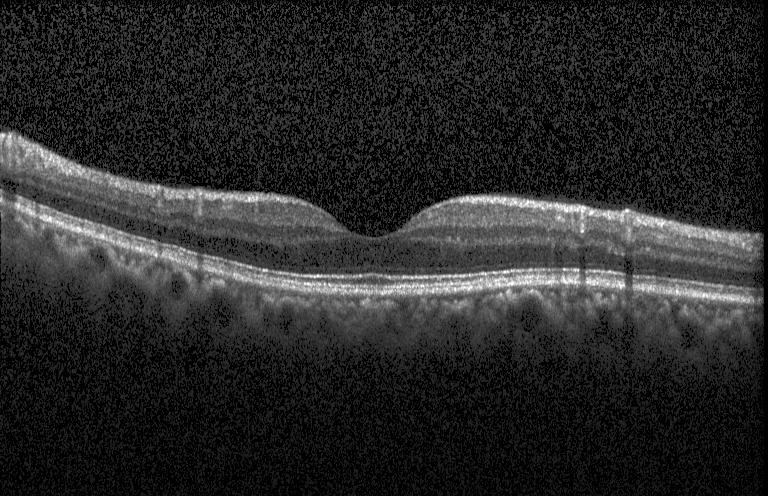
Optical coherence tomography B-scan, centered on the fovea, Heidelberg Spectralis.
OCT finding: no choroidal neovascularization, no diabetic macular edema, and no drusen.